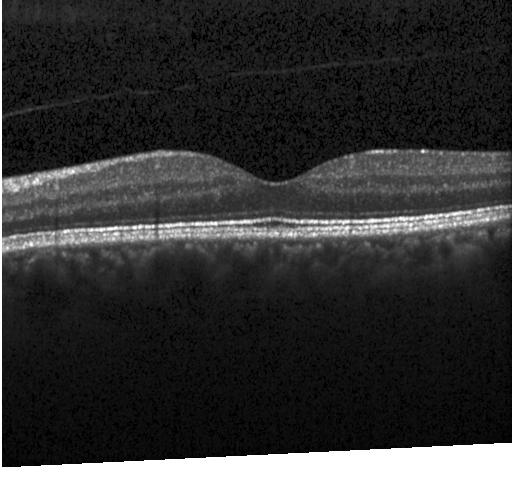

Assessment: neither choroidal neovascularization, diabetic macular edema, nor drusen.